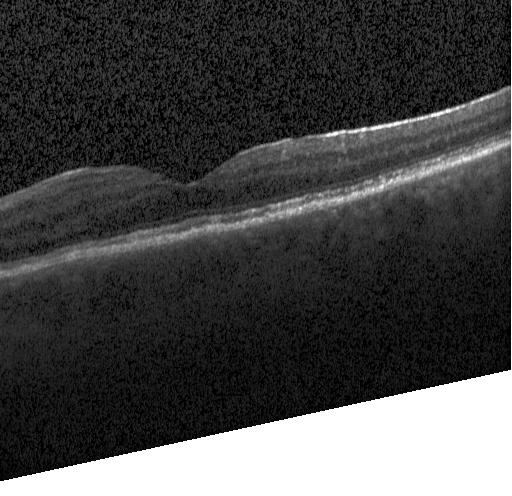
SD-OCT; OCT line scan — OCT finding: no choroidal neovascularization, no diabetic macular edema, and no drusen.